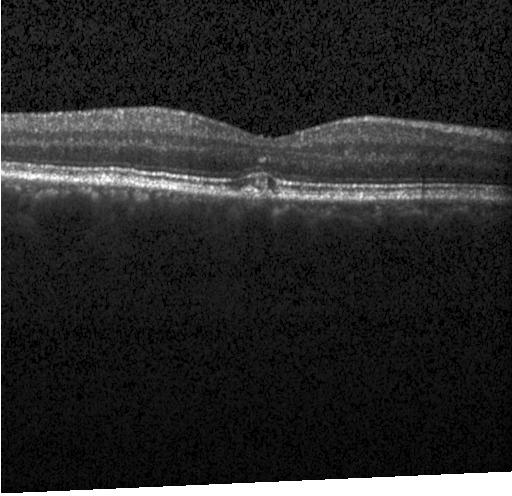
Horizontal scan through the fovea. Spectral-domain optical coherence tomography. OCT line scan. Acquired on a Heidelberg Spectralis
Diagnosis: drusen.